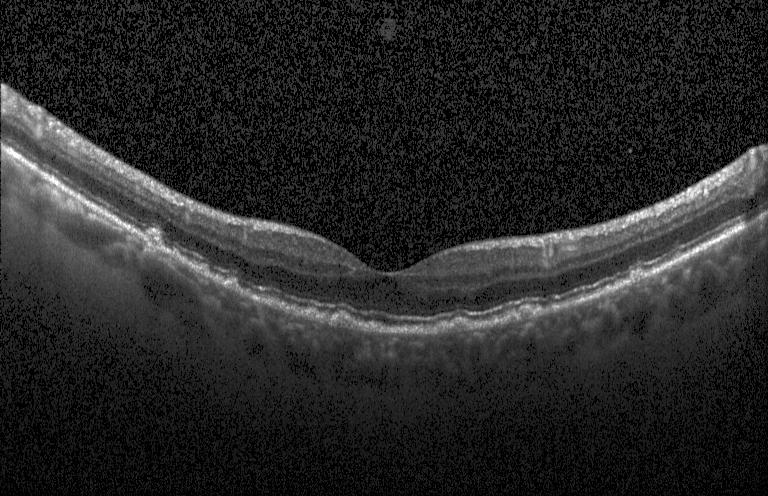

OCT finding: sub-RPE drusenoid deposits.